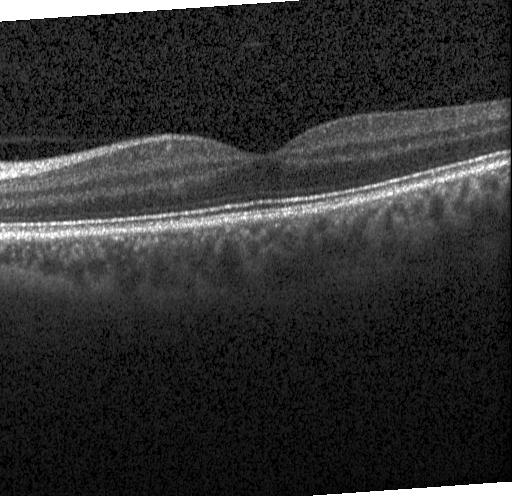

OCT line scan. OCT finding: no choroidal neovascularization, no diabetic macular edema, and no drusen.